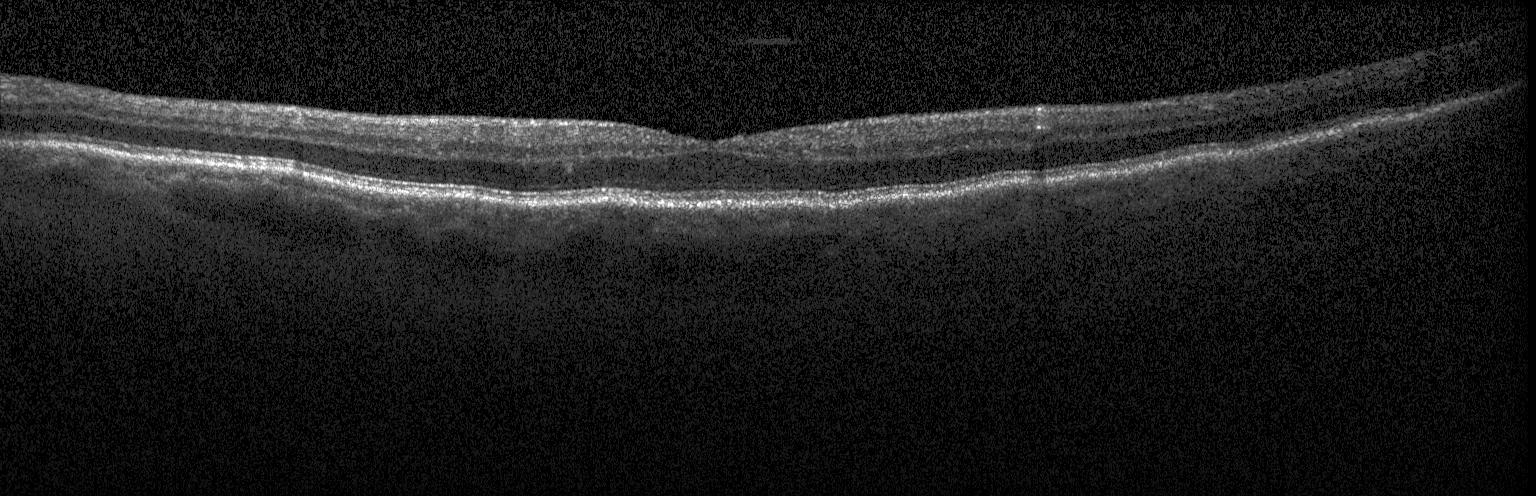
Retinal OCT cross-section
Diagnosis: no CNV, no DME, and no drusen.